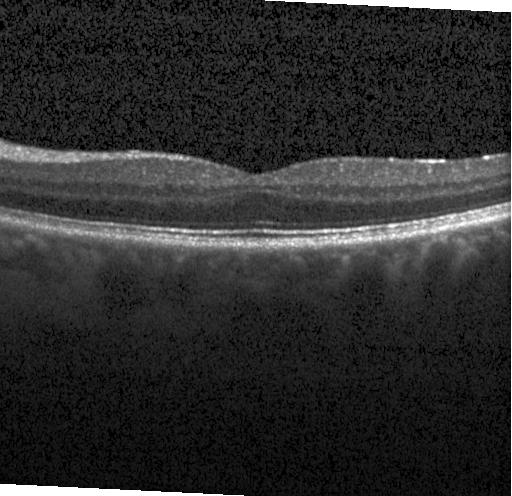 Retinal OCT cross-section — The scan shows no choroidal neovascularization, diabetic macular edema, or drusen.